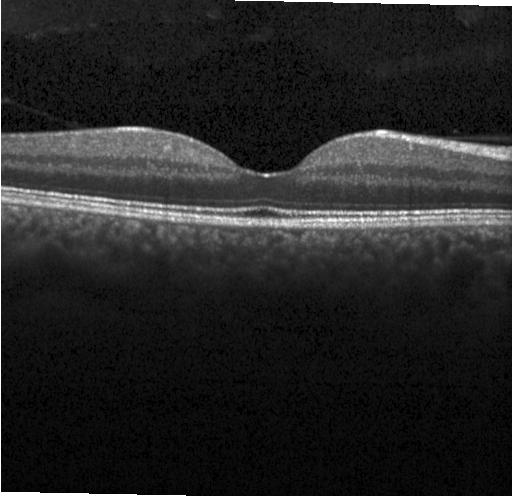
Optical coherence tomography scan; spectral-domain OCT; macular scan. Assessment: no choroidal neovascularization, no diabetic macular edema, and no drusen.